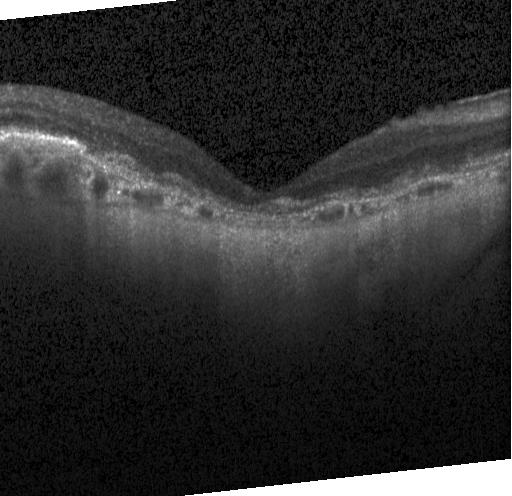 OCT line scan. Instrument: Heidelberg Spectralis. SD-OCT. Centered on the fovea. Macular OCT: a choroidal neovascular membrane.